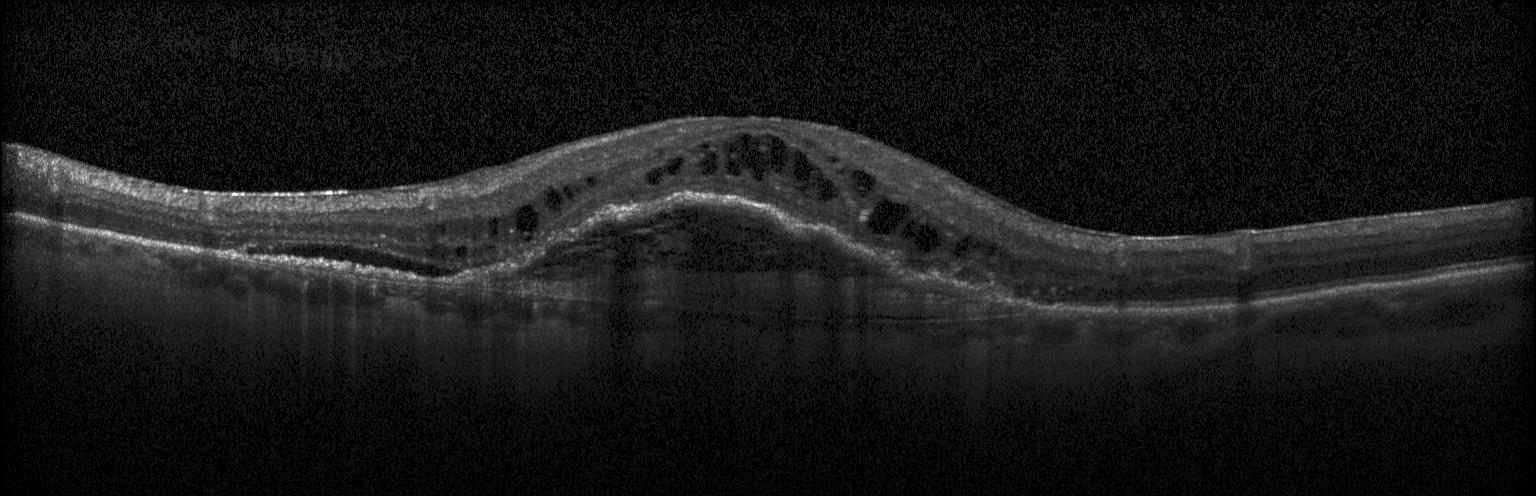

Optical coherence tomography B-scan, spectral-domain OCT, through the macula — Diagnosis: choroidal neovascularization (CNV).